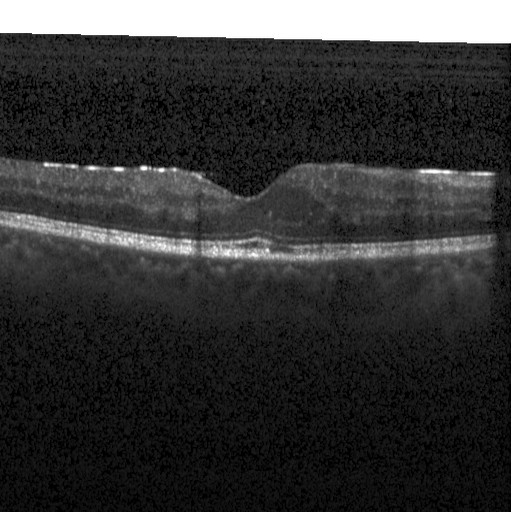 Diagnosis: DME.